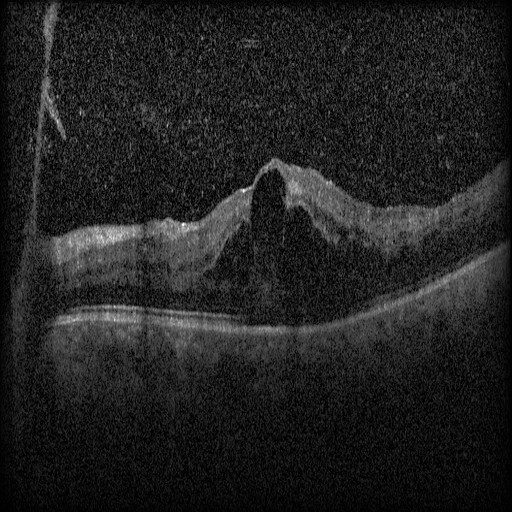
Macular OCT: diabetic macular edema.